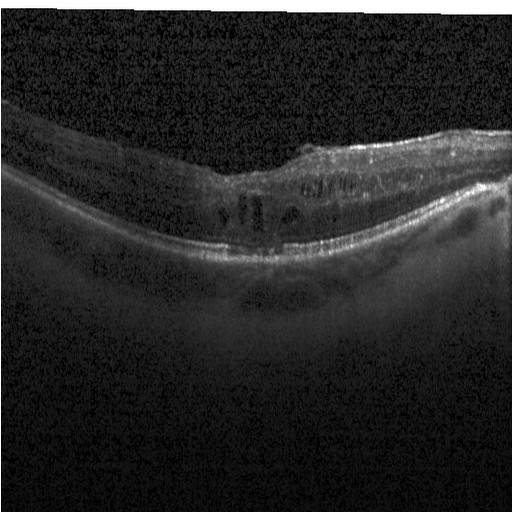

Optical coherence tomography B-scan — Impression: DME.